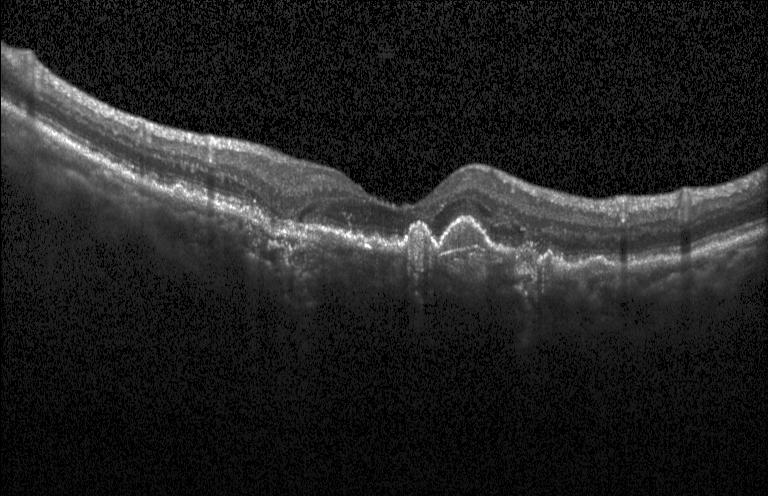 This B-scan demonstrates choroidal neovascularization (CNV).